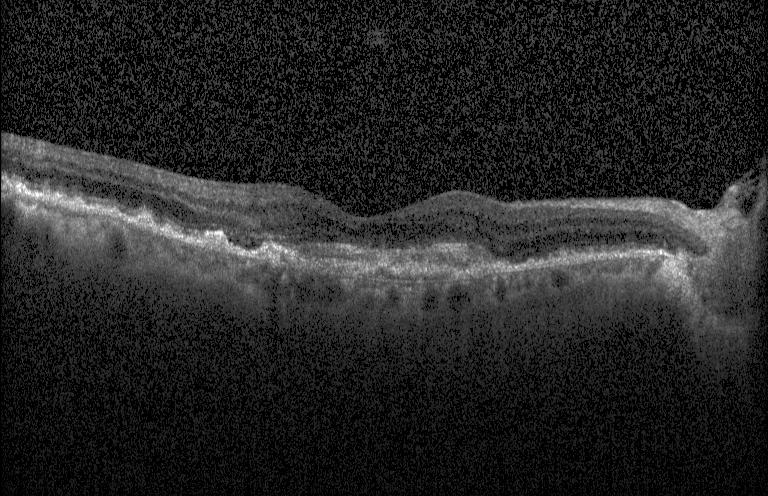 Optical coherence tomography B-scan. Heidelberg Spectralis. This B-scan demonstrates choroidal neovascularization.